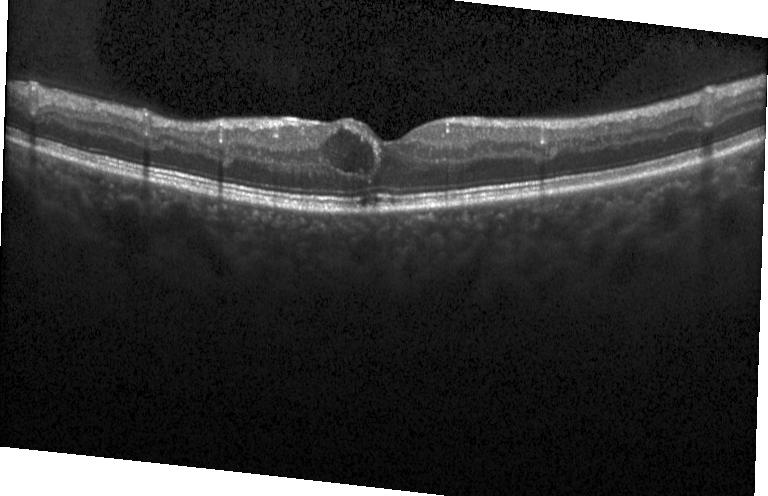
Spectral-domain optical coherence tomography. Horizontal scan through the fovea. Heidelberg Spectralis OCT system. OCT B-scan — Diabetic macular edema.